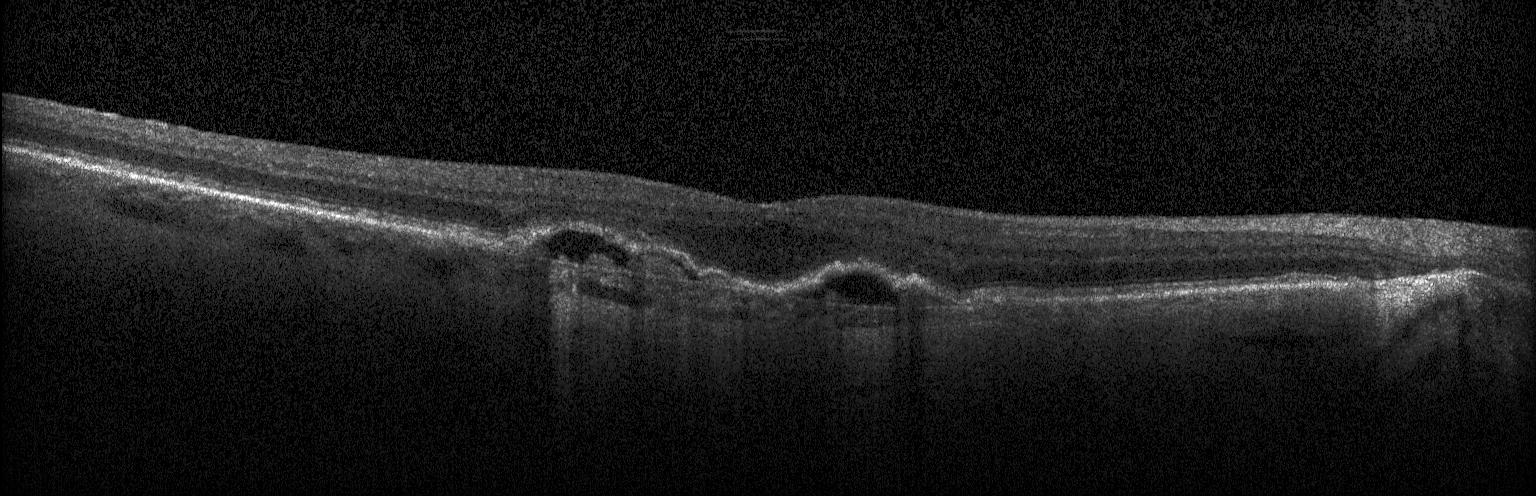

Macular scan, OCT line scan.
Diagnosis: a choroidal neovascular membrane.